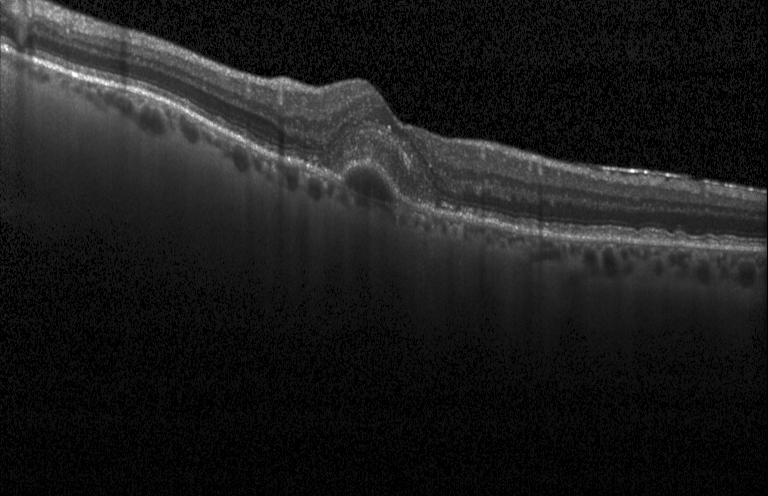

OCT B-scan · spectral-domain OCT — This B-scan demonstrates a choroidal neovascular membrane.